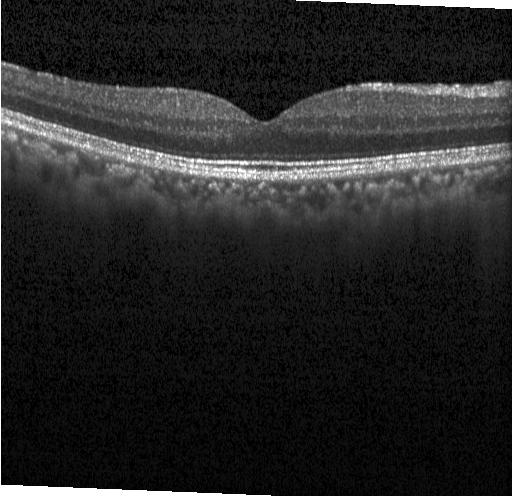

Centered on the fovea; OCT B-scan — OCT finding: no evidence of CNV, DME, or drusen.